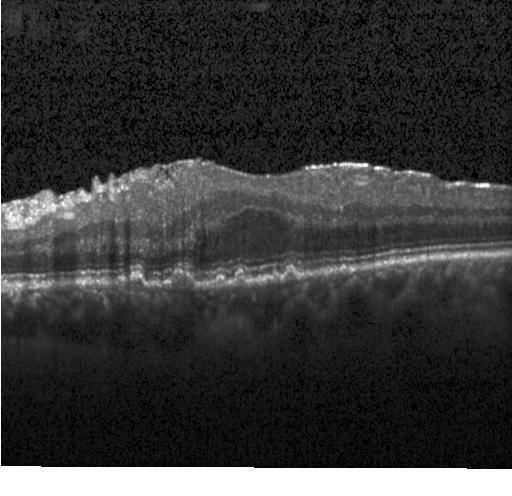
Diagnosis: sub-RPE drusenoid deposits.